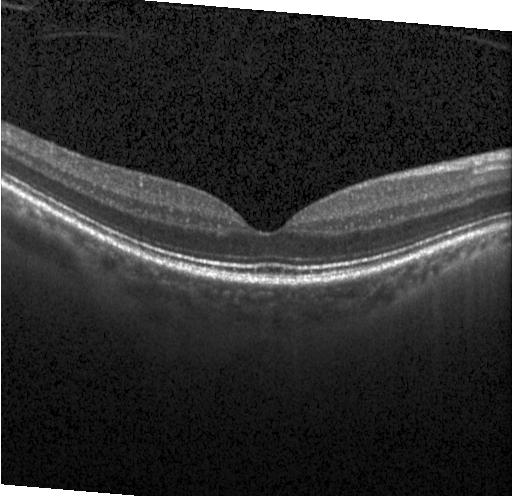 OCT B-scan showing no evidence of CNV, DME, or drusen.